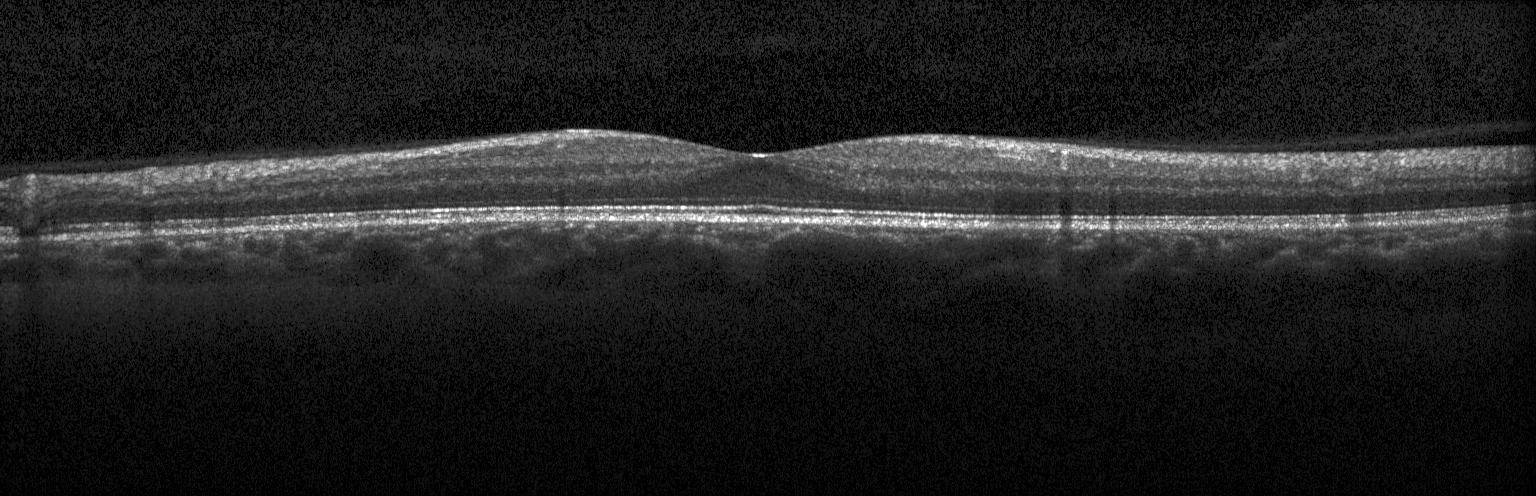
Optical coherence tomography B-scan — Diagnosis: no CNV, DME, or drusen.